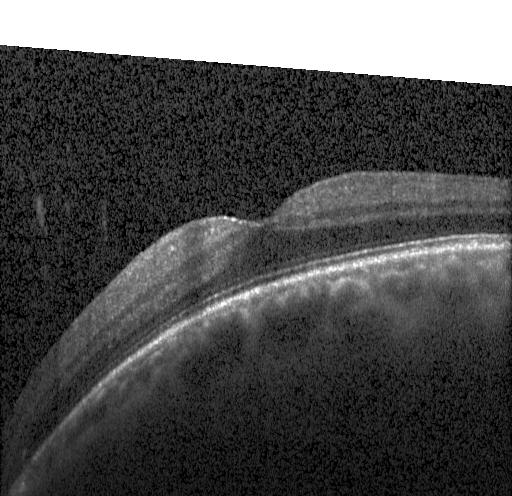

Diagnosis: neither choroidal neovascularization, diabetic macular edema, nor drusen.